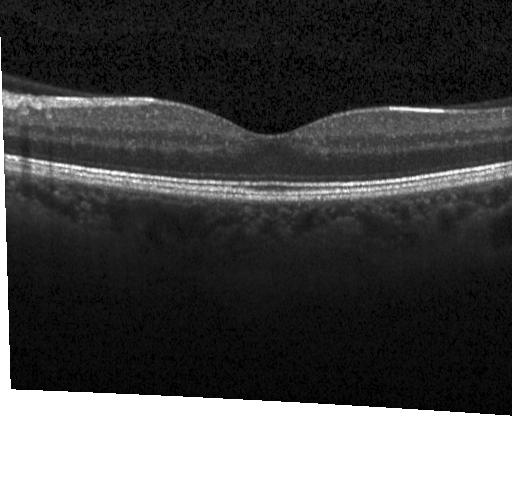
Retinal OCT cross-section. Heidelberg Spectralis. Finding: neither CNV, DME, nor drusen.